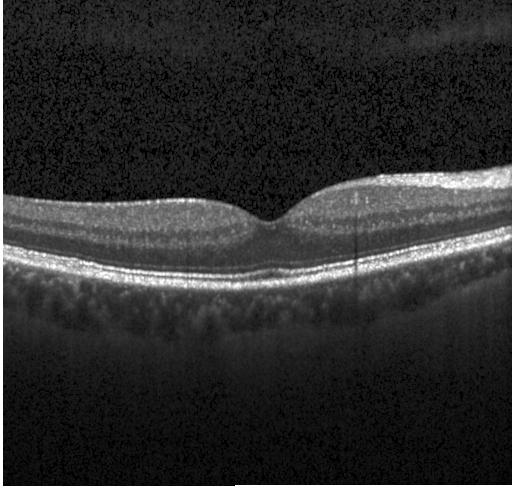

Finding: no evidence of choroidal neovascularization, diabetic macular edema, or drusen.